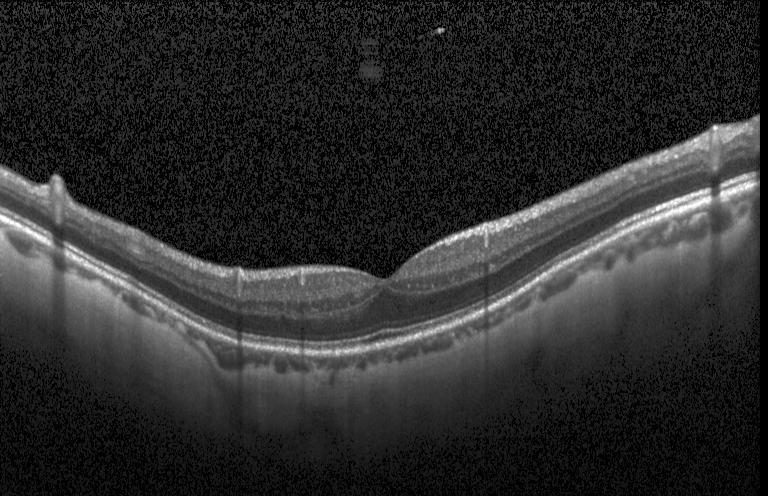

OCT line scan, instrument: Heidelberg Spectralis, horizontal scan through the fovea, spectral-domain OCT
Macular OCT: no CNV, DME, or drusen.